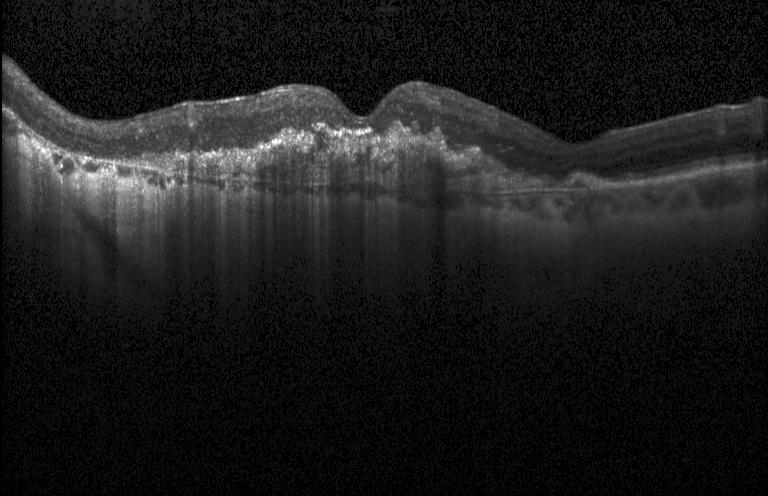
OCT B-scan, acquired on a Heidelberg Spectralis, spectral-domain OCT.
Finding: a choroidal neovascular membrane.